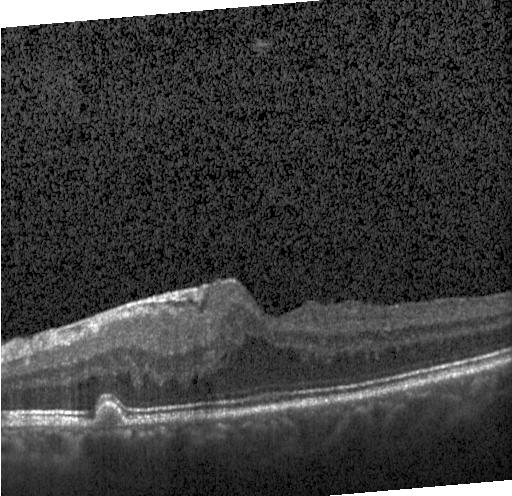 Acquired on a Heidelberg Spectralis; OCT B-scan; spectral-domain optical coherence tomography; horizontal scan through the fovea
OCT finding: multiple drusen.